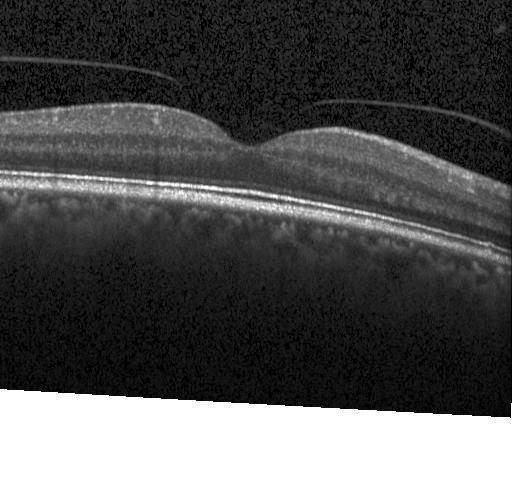

Spectral-domain OCT B-scan: no evidence of CNV, DME, or drusen.